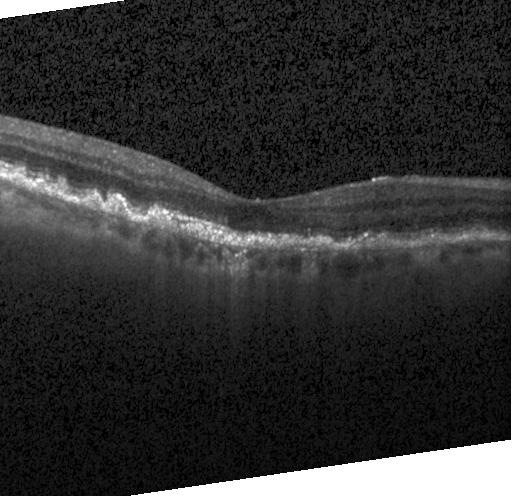

Spectral-domain OCT B-scan: choroidal neovascularization (CNV).